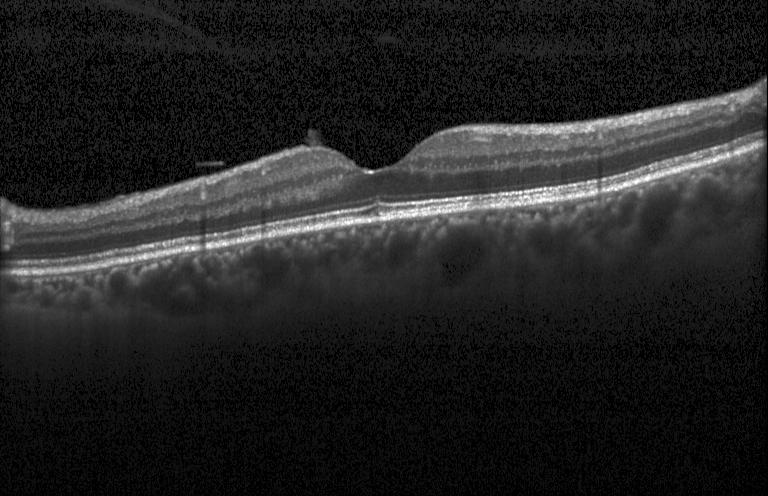
Finding: no CNV, DME, or drusen.